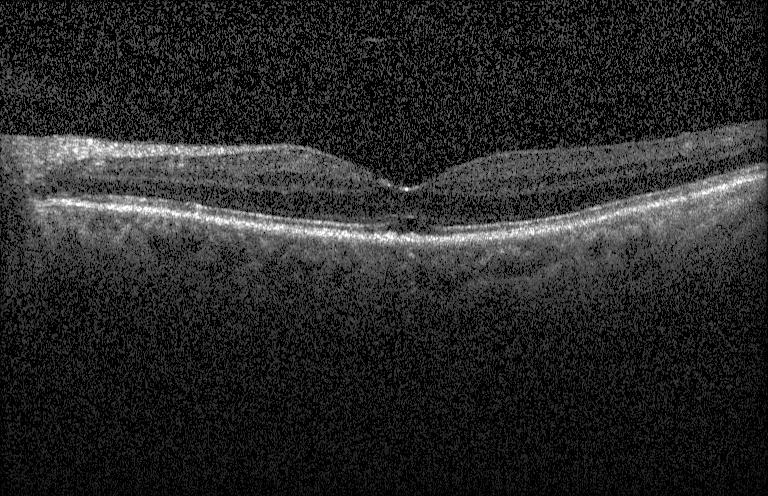 Impression: no choroidal neovascularization, no diabetic macular edema, and no drusen.